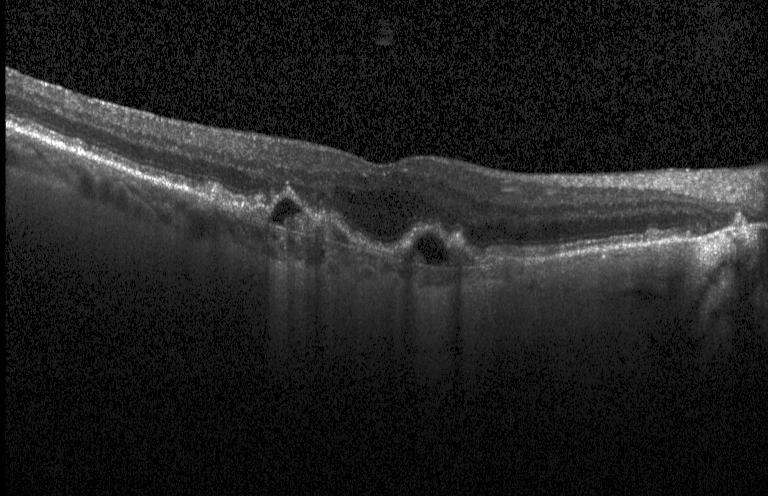

OCT B-scan · SD-OCT — Finding: choroidal neovascularization (CNV).